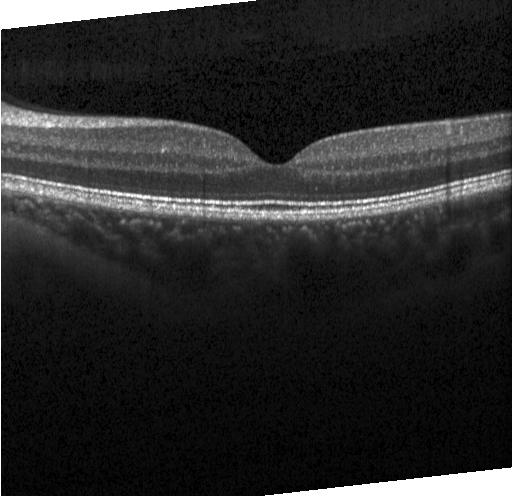

Finding: neither choroidal neovascularization, diabetic macular edema, nor drusen.